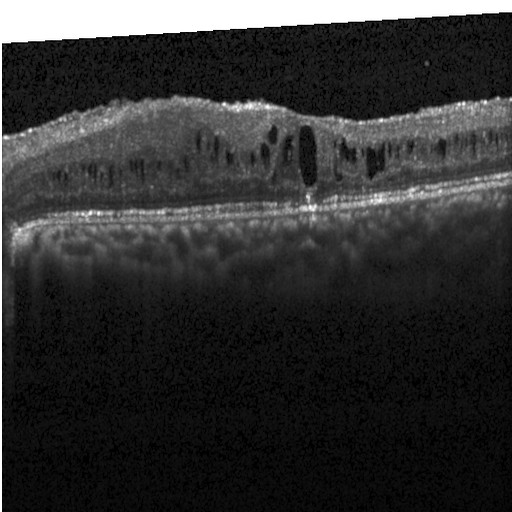 Retinal OCT B-scan — Assessment: diabetic macular edema (DME).